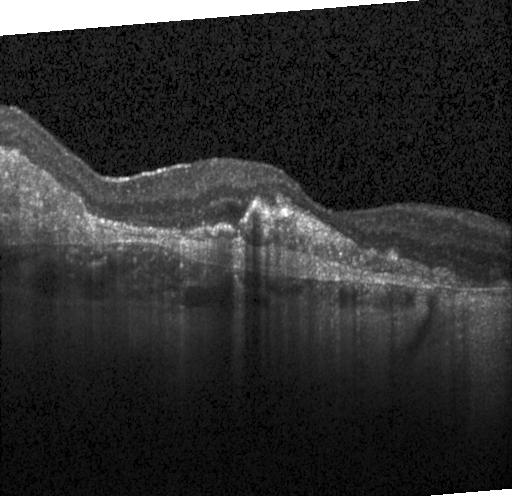 Spectral-domain optical coherence tomography · instrument: Heidelberg Spectralis · OCT line scan · macular scan — Impression: a choroidal neovascular membrane.